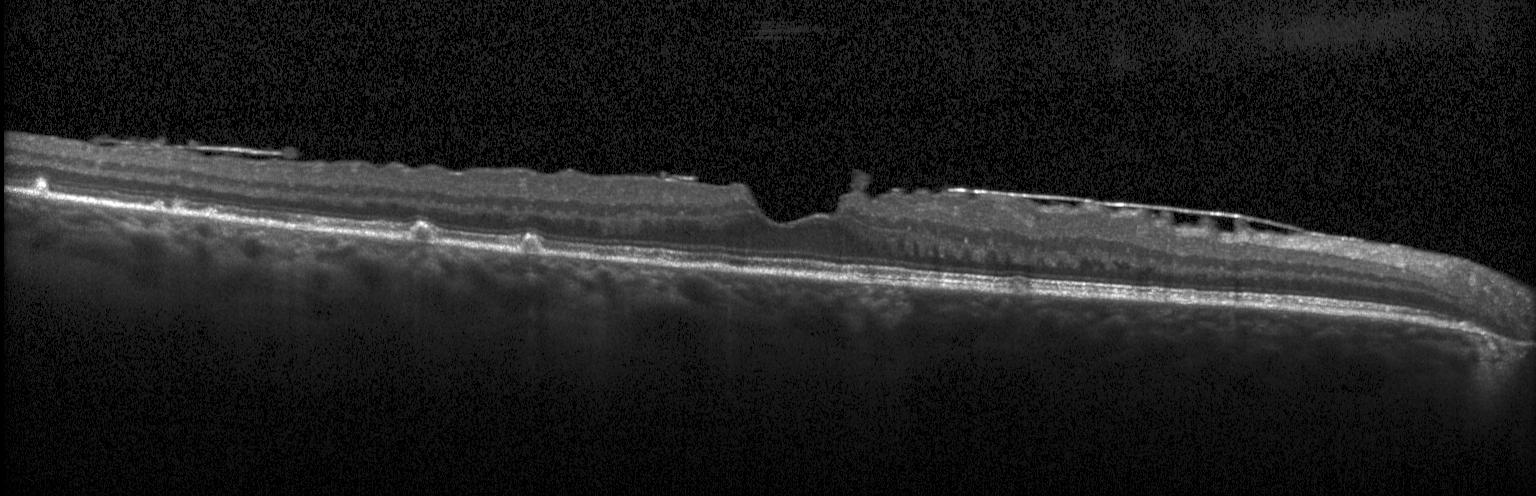

This B-scan demonstrates multiple drusen.